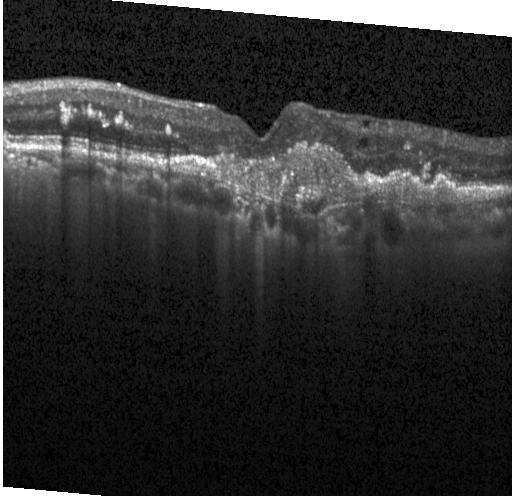 Retinal OCT cross-section showing CNV.